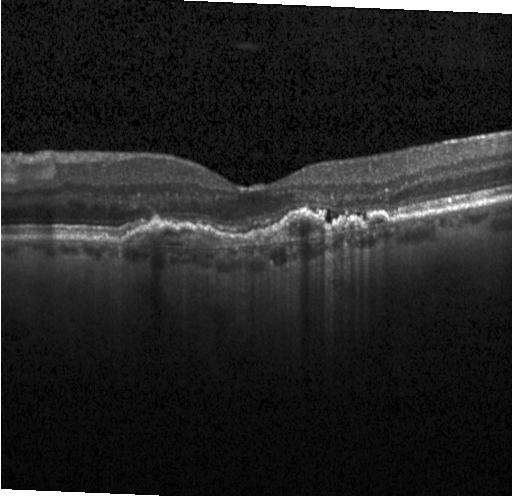

Retinal OCT B-scan, SD-OCT. Diagnosis: choroidal neovascularization.